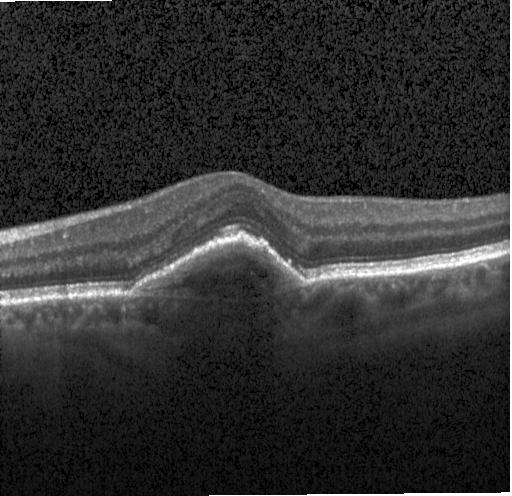 Retinal OCT B-scan. Macular OCT: choroidal neovascularization (CNV).